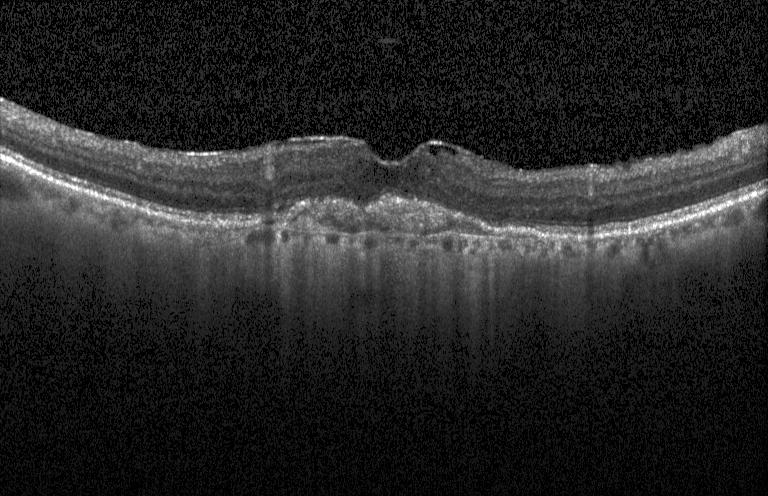 OCT B-scan. Centered on the fovea
Finding: a choroidal neovascular membrane.